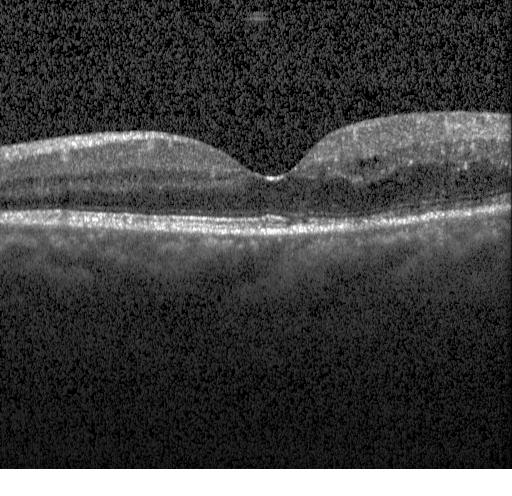
Retinal OCT B-scan
Dx: DME.